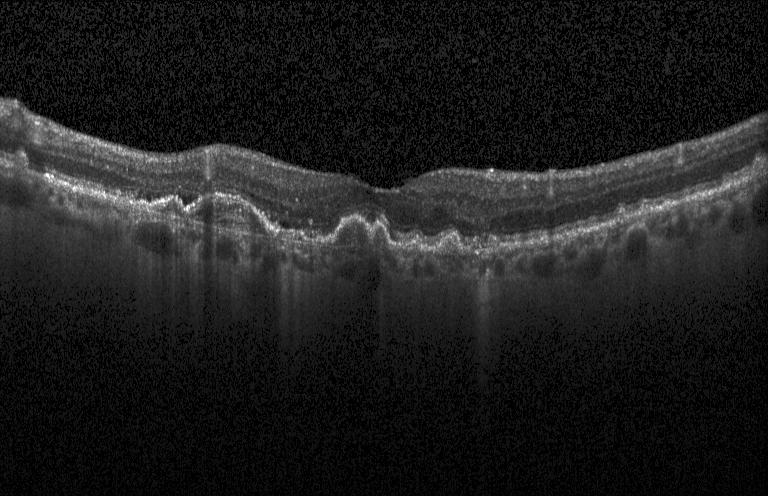

OCT B-scan showing choroidal neovascularization (CNV).